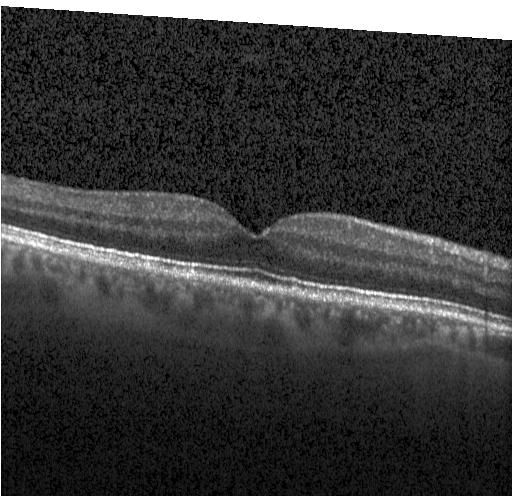

Through the macula, SD-OCT, retinal OCT B-scan.
Diagnosis: no CNV, DME, or drusen.